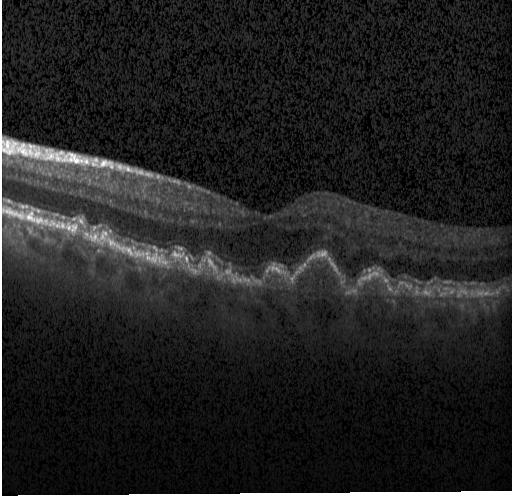 Spectral-domain OCT; OCT line scan; macular scan
OCT finding: multiple drusen.